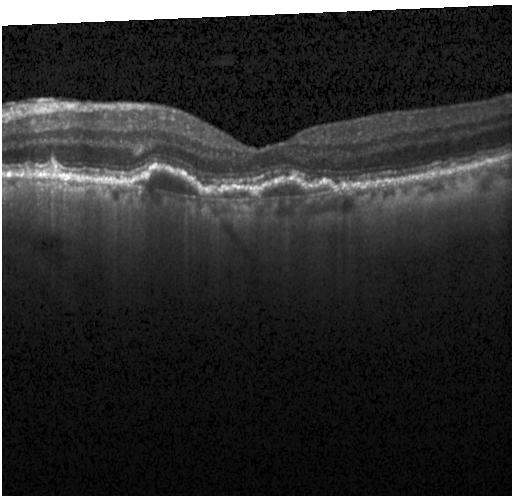

Diagnosis: CNV.